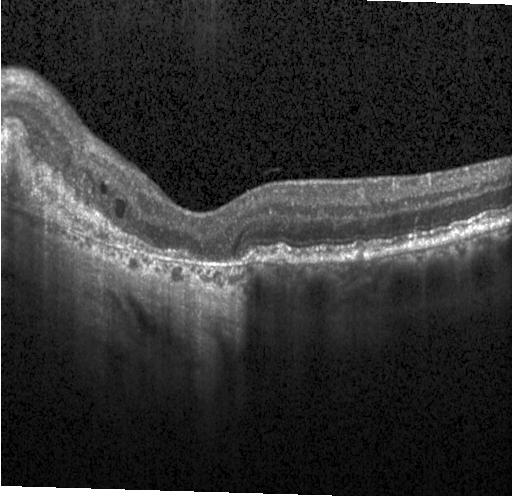

Retinal OCT cross-section, centered on the fovea, instrument: Heidelberg Spectralis, spectral-domain OCT
Diagnosis: choroidal neovascularization (CNV).